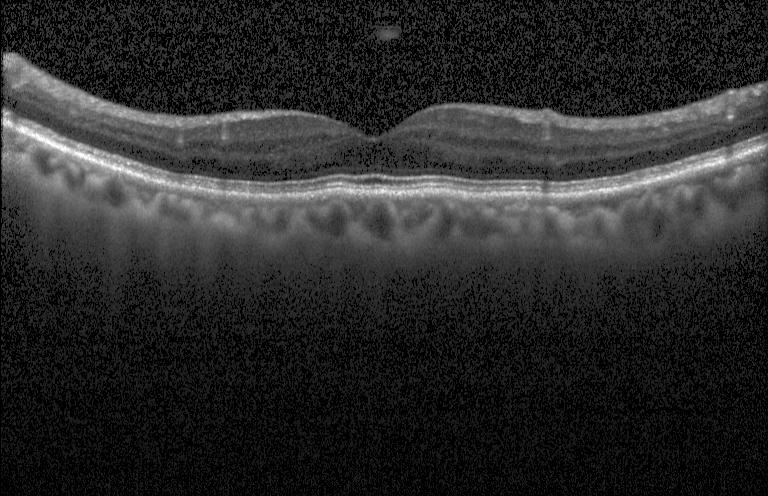
Diagnosis: neither CNV, DME, nor drusen.